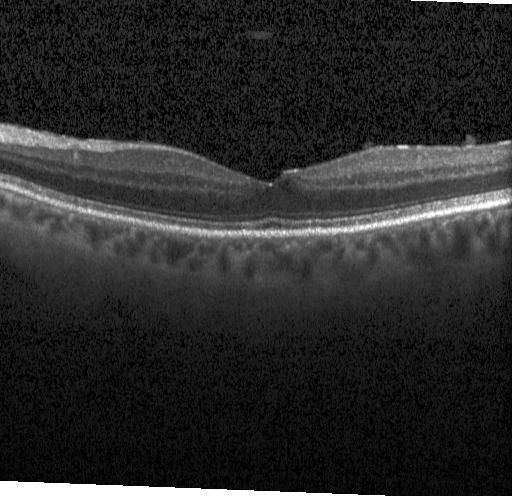 Heidelberg Spectralis; retinal OCT cross-section; horizontal scan through the fovea. Finding: no evidence of choroidal neovascularization, diabetic macular edema, or drusen.